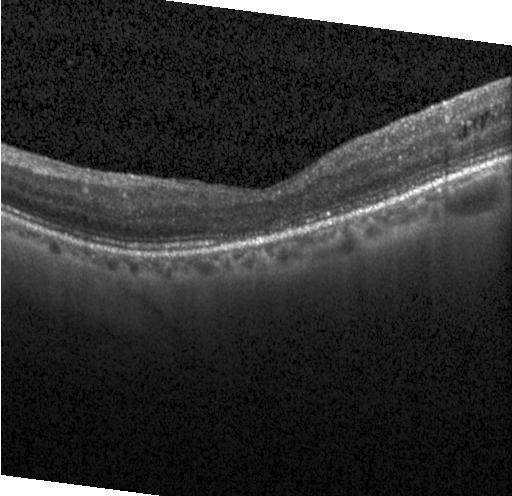
Optical coherence tomography B-scan.
Diabetic macular edema.